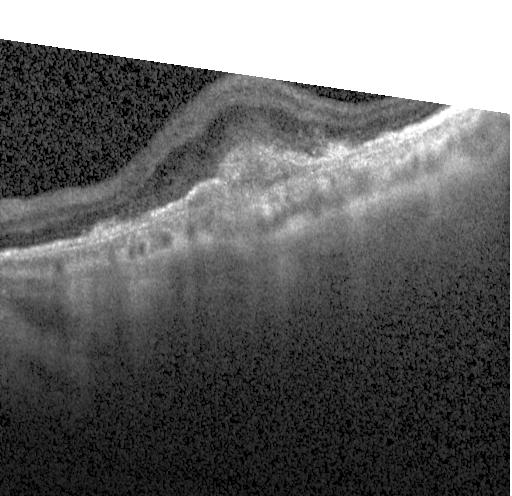 Impression: choroidal neovascularization.